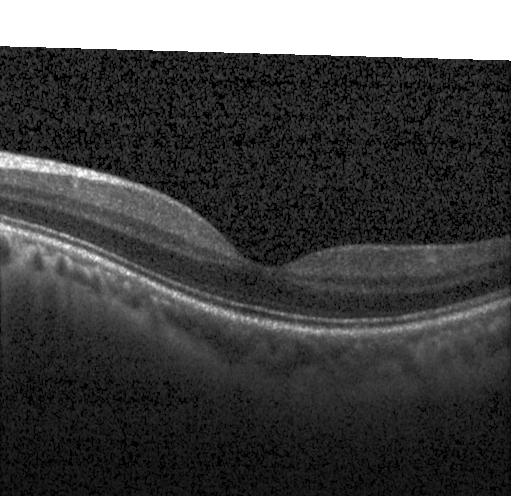
Macular OCT: no evidence of choroidal neovascularization, diabetic macular edema, or drusen.